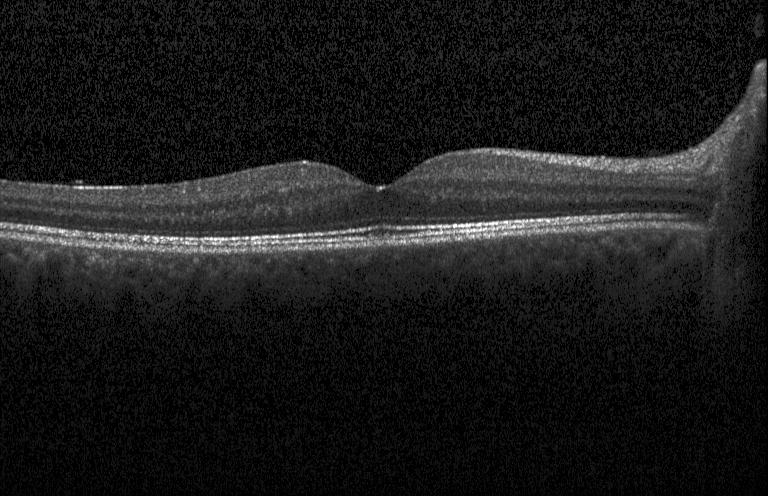 Assessment: no evidence of choroidal neovascularization, diabetic macular edema, or drusen.